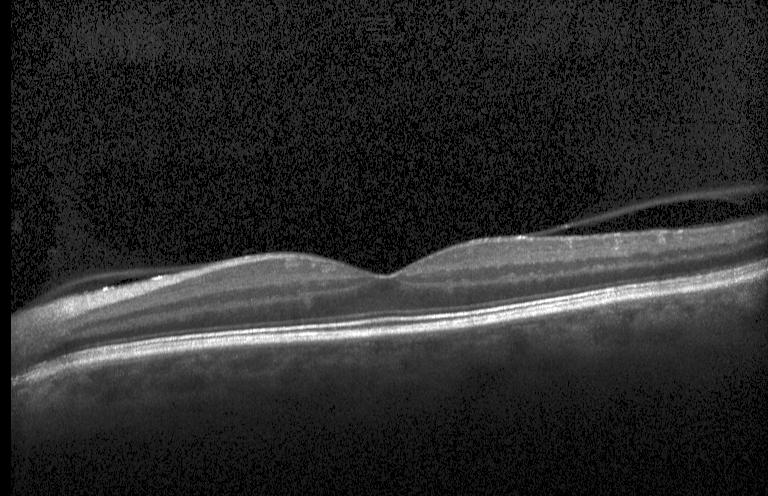

Optical coherence tomography scan
Assessment: neither choroidal neovascularization, diabetic macular edema, nor drusen.